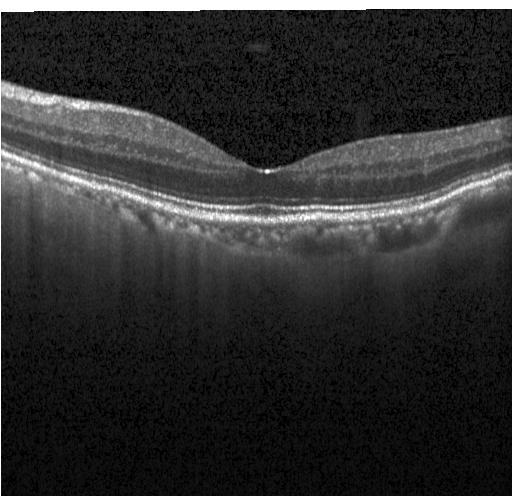

OCT line scan — Assessment: neither choroidal neovascularization, diabetic macular edema, nor drusen.